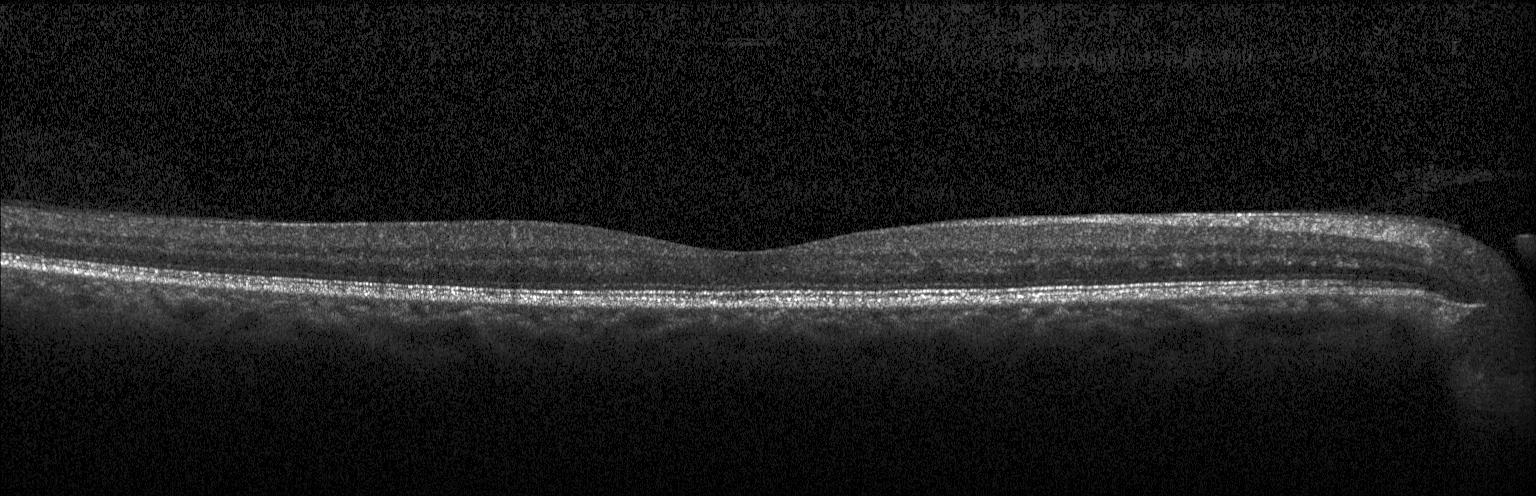
OCT line scan.
Impression: no evidence of choroidal neovascularization, diabetic macular edema, or drusen.